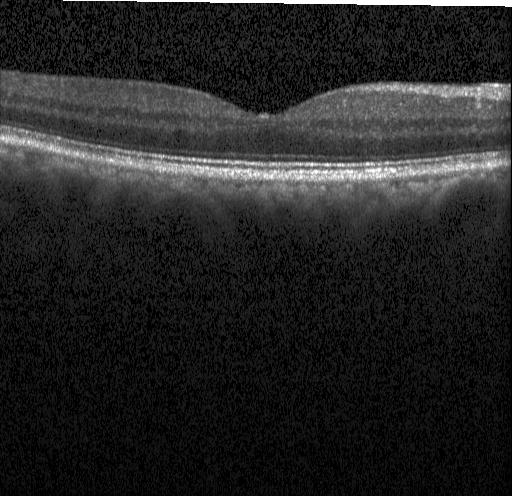 Neither choroidal neovascularization, diabetic macular edema, nor drusen.